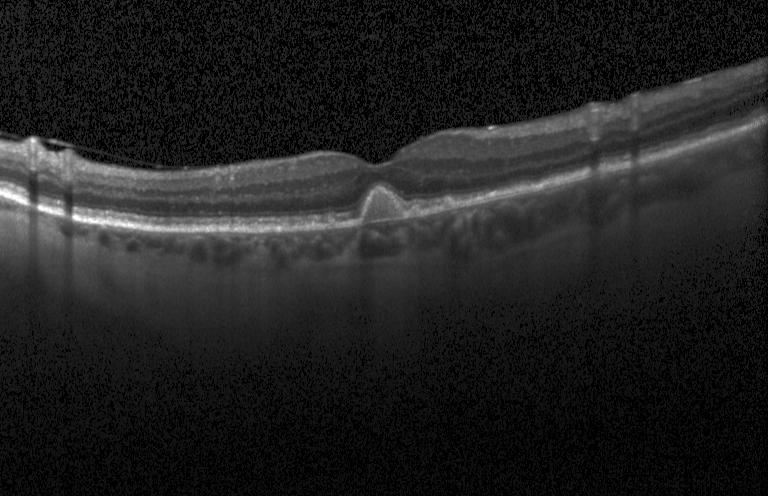 Optical coherence tomography B-scan
Impression: multiple drusen.